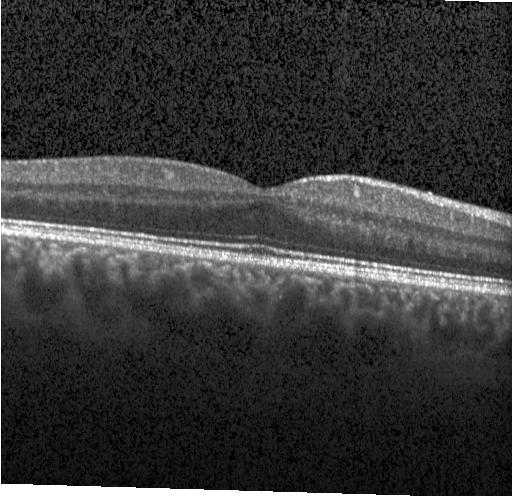

Impression: neither choroidal neovascularization, diabetic macular edema, nor drusen.